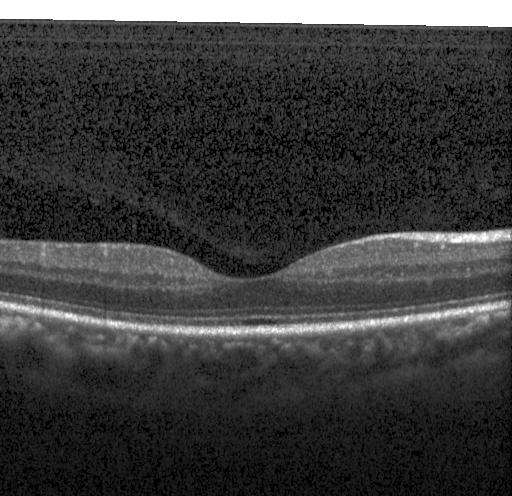
Macular scan · spectral-domain optical coherence tomography · OCT line scan.
Finding: neither choroidal neovascularization, diabetic macular edema, nor drusen.